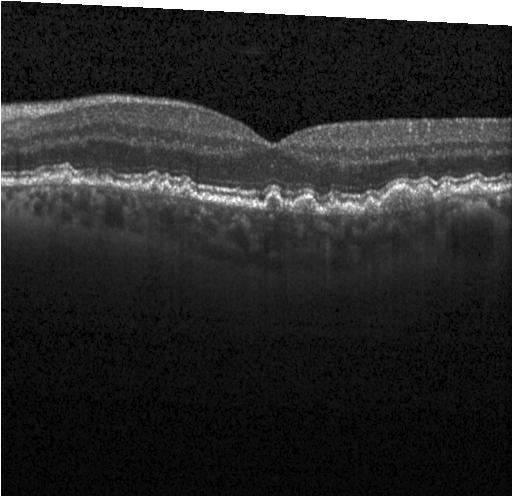 Heidelberg Spectralis OCT system. Retinal OCT B-scan. Spectral-domain OCT
Diagnosis: multiple drusen.